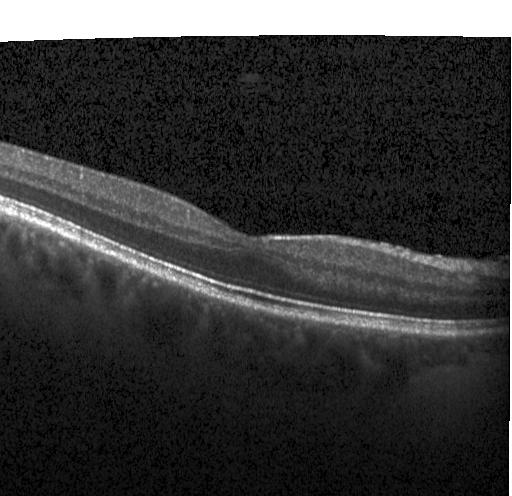

OCT line scan. Heidelberg Spectralis OCT system. Through the macula. Impression: no choroidal neovascularization, no diabetic macular edema, and no drusen.